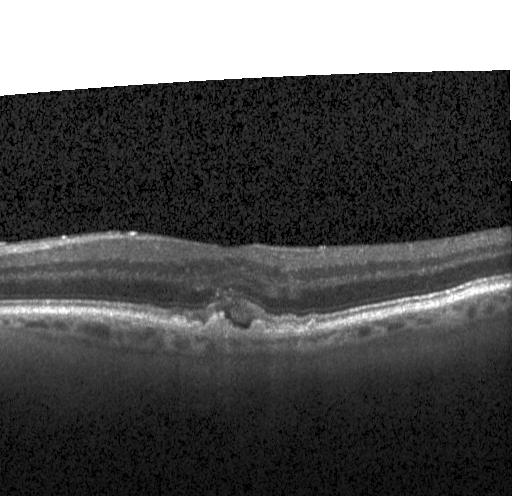 OCT B-scan. Dx: CNV.